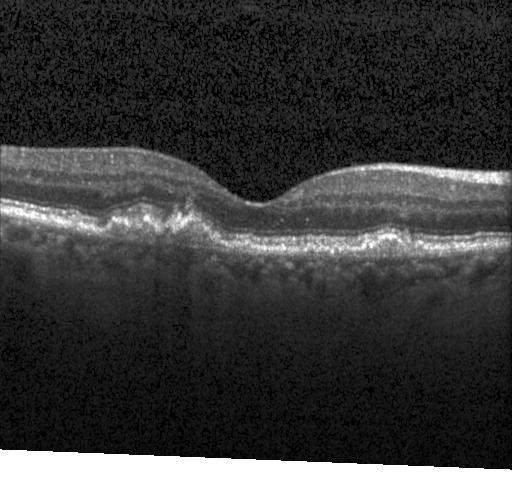
Optical coherence tomography scan
Assessment: a choroidal neovascular membrane.